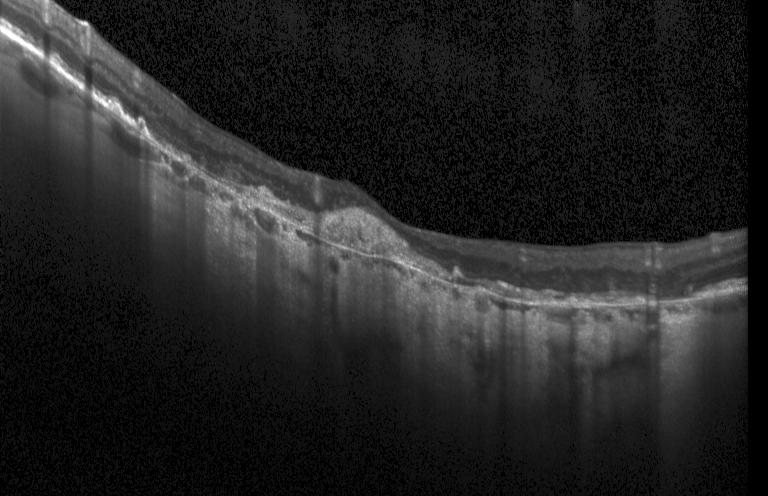
SD-OCT · through the macula · retinal OCT cross-section — Macular OCT: a choroidal neovascular membrane.